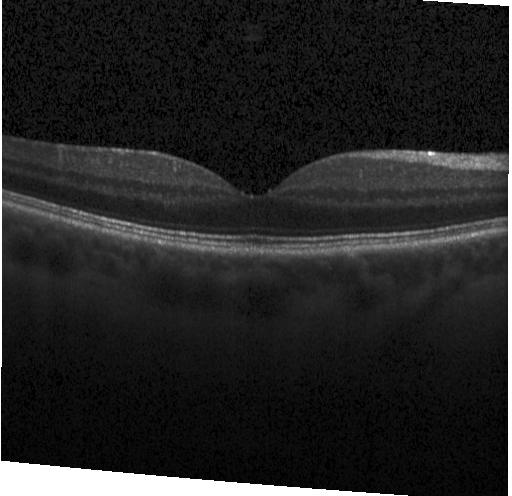
Diagnosis: neither choroidal neovascularization, diabetic macular edema, nor drusen.